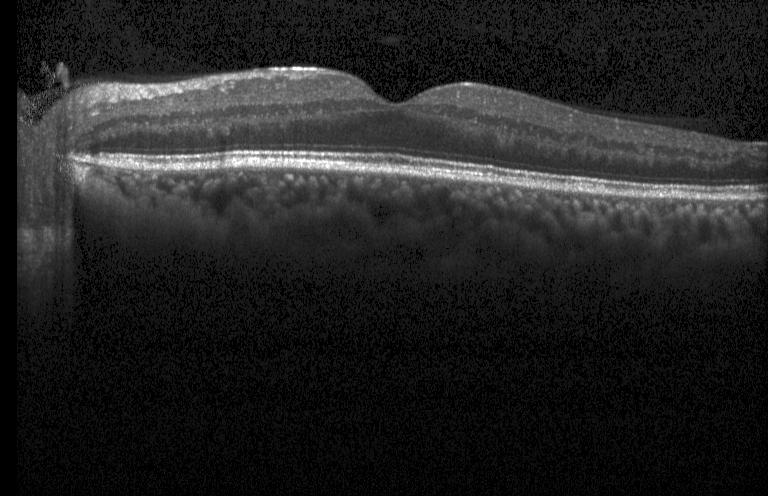

Heidelberg Spectralis OCT system. Optical coherence tomography scan
The scan shows neither CNV, DME, nor drusen.